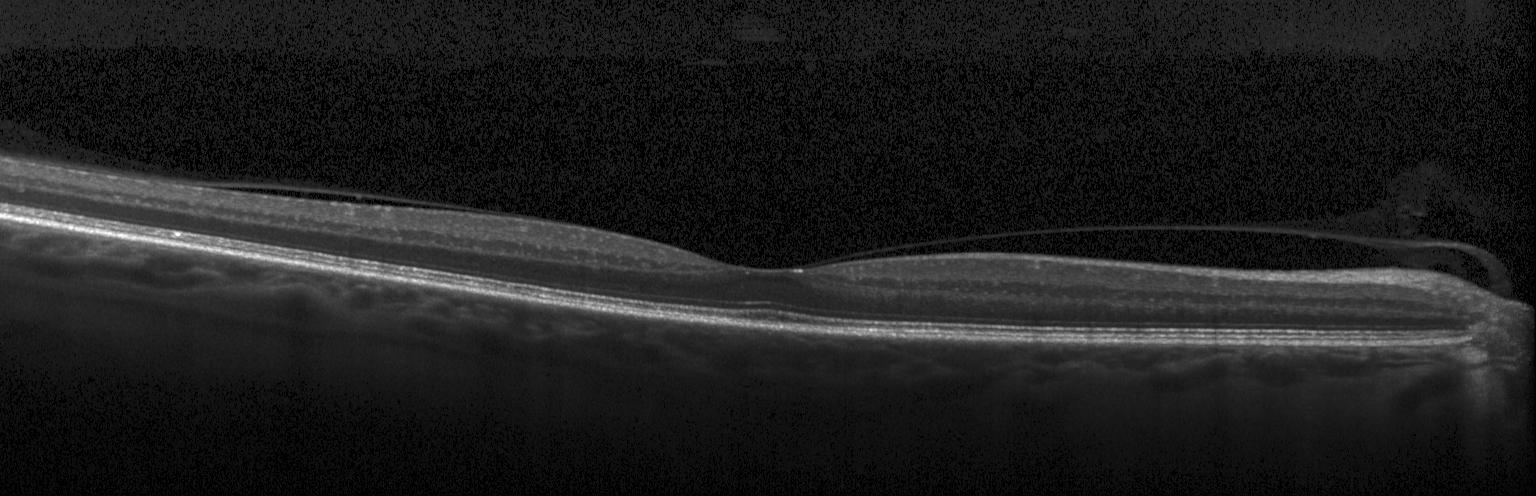

Finding: neither CNV, DME, nor drusen.